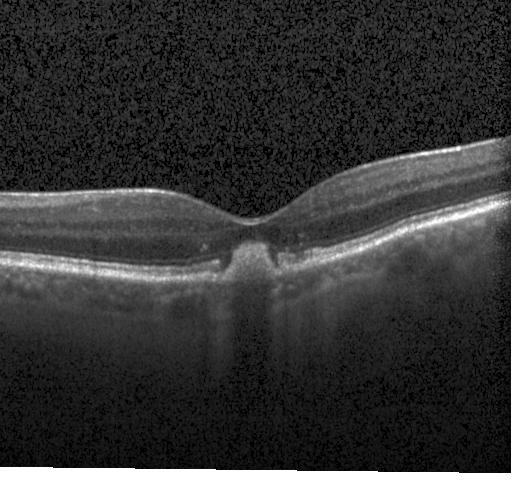 Instrument: Heidelberg Spectralis · optical coherence tomography B-scan · horizontal scan through the fovea — Impression: choroidal neovascularization.